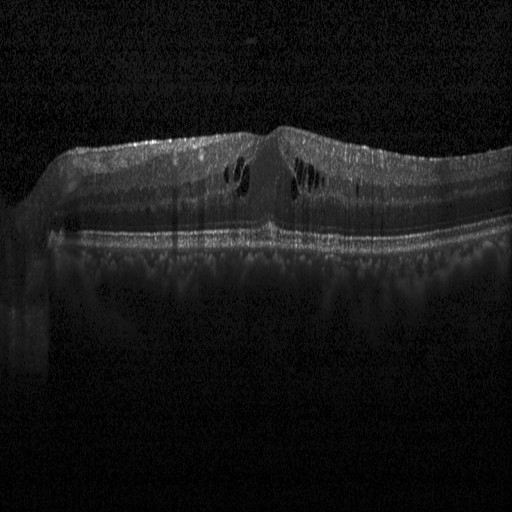 Optical coherence tomography scan.
The scan shows DME.